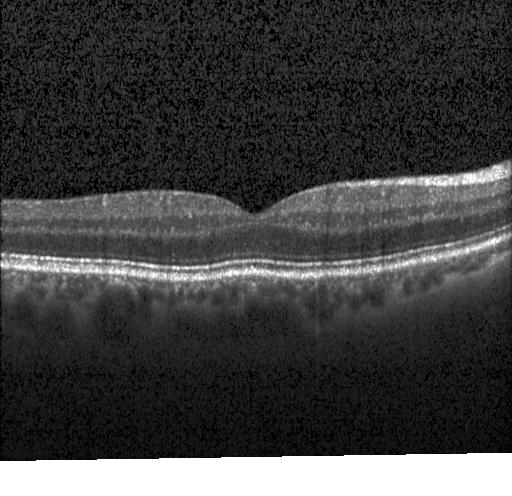 Retinal OCT cross-section · spectral-domain optical coherence tomography · horizontal scan through the fovea · acquired on a Heidelberg Spectralis — Diagnosis: neither CNV, DME, nor drusen.